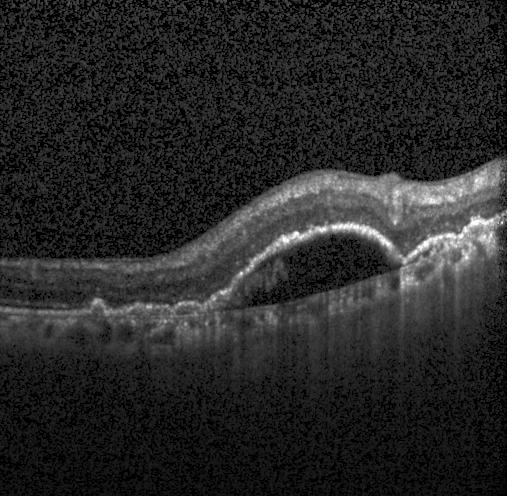 Finding: a choroidal neovascular membrane.